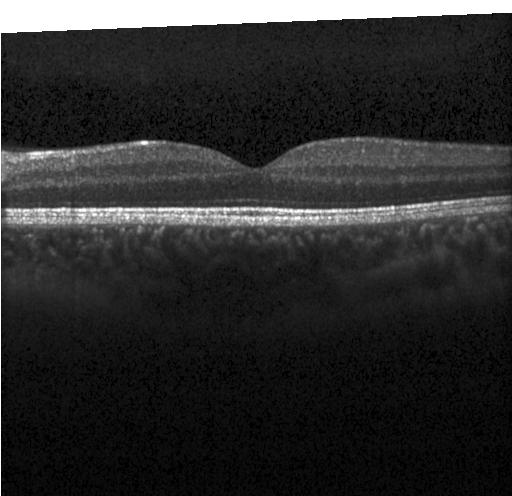
Impression: neither choroidal neovascularization, diabetic macular edema, nor drusen.